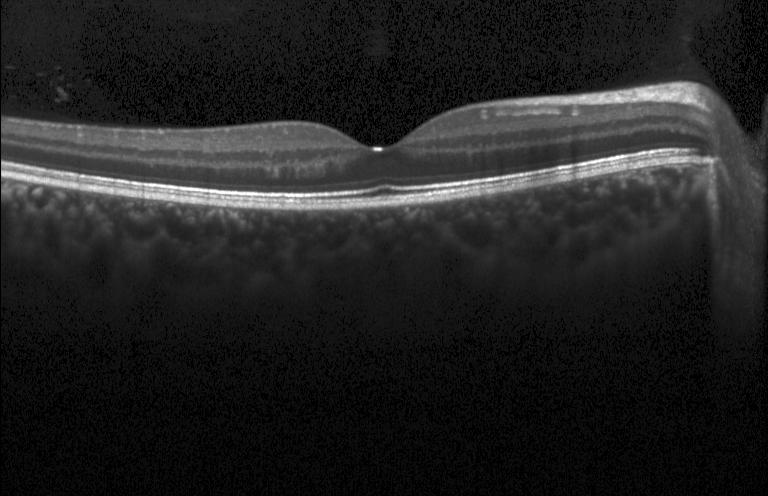

Dx: no evidence of choroidal neovascularization, diabetic macular edema, or drusen.